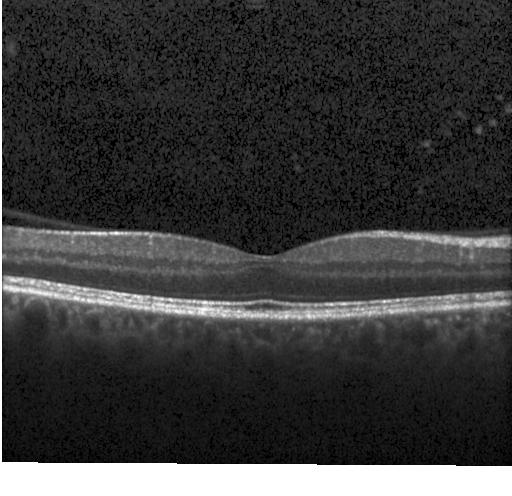

OCT B-scan showing no evidence of choroidal neovascularization, diabetic macular edema, or drusen.